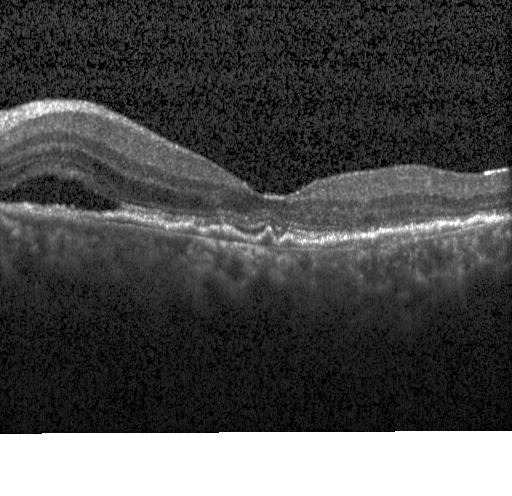
OCT scan showing a choroidal neovascular membrane.